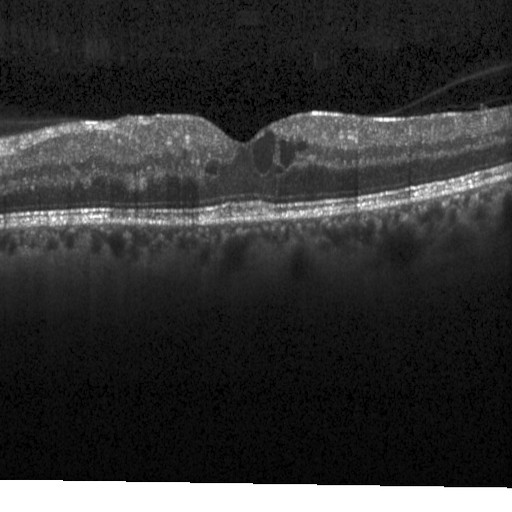

Horizontal scan through the fovea. Heidelberg Spectralis. OCT B-scan. SD-OCT — Diagnosis: DME.